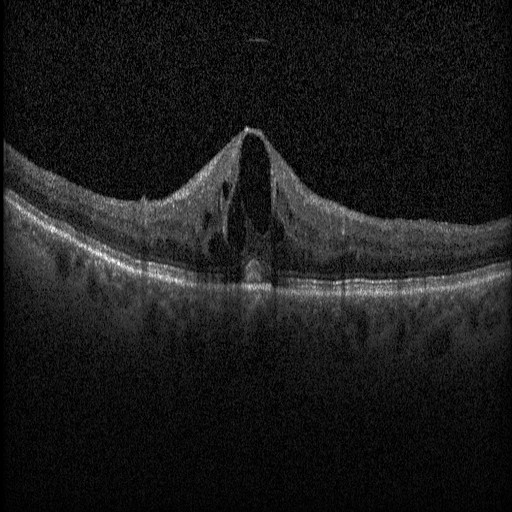
Diabetic macular edema (DME).